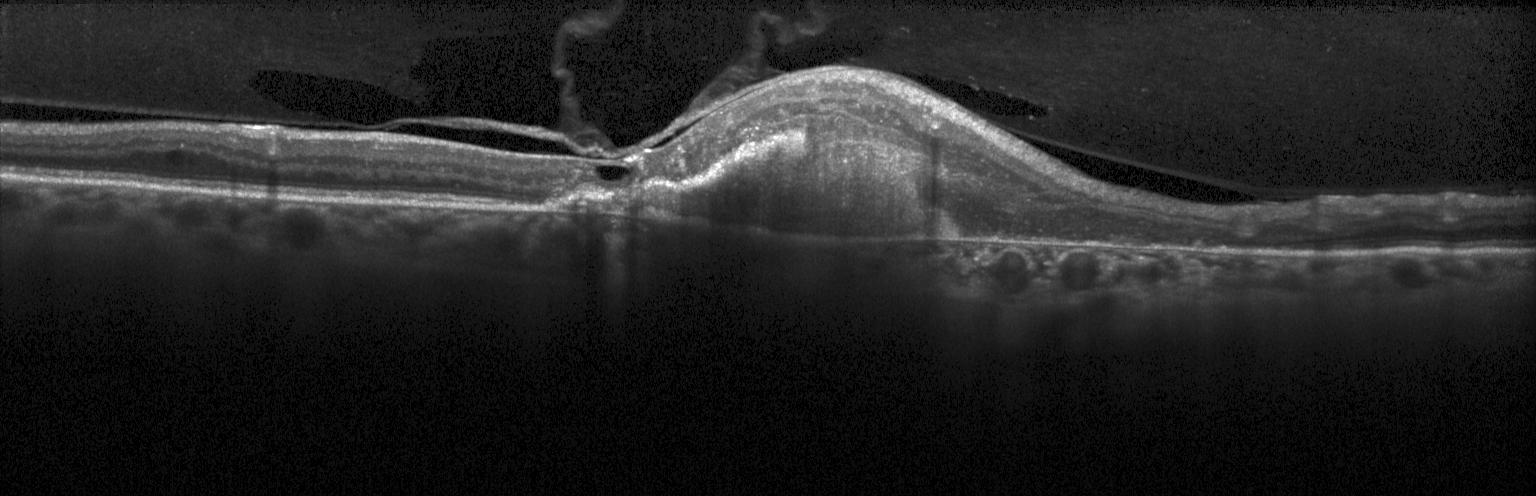
Retinal OCT B-scan. Impression: a choroidal neovascular membrane.